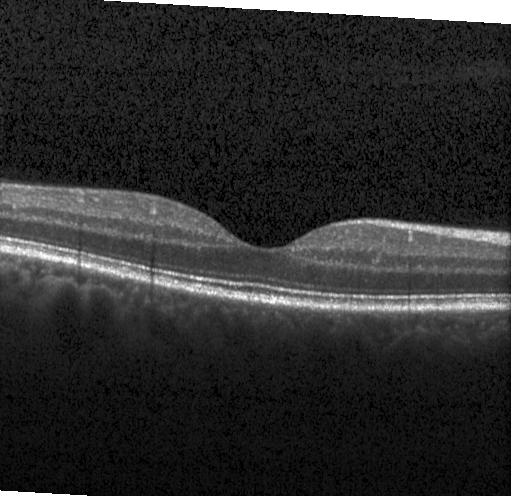

Heidelberg Spectralis OCT system, optical coherence tomography scan, SD-OCT — No choroidal neovascularization, no diabetic macular edema, and no drusen.